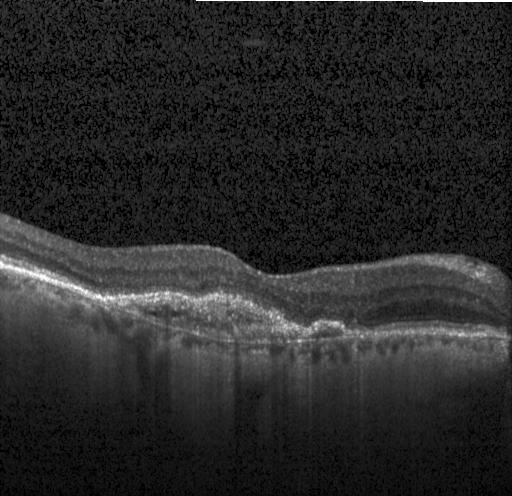

Spectral-domain optical coherence tomography; through the macula; retinal OCT cross-section. Assessment: choroidal neovascularization (CNV).